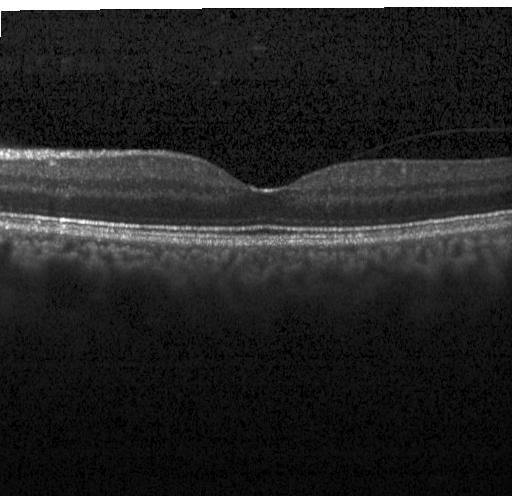

SD-OCT, OCT line scan, through the macula, Heidelberg Spectralis.
Finding: no evidence of CNV, DME, or drusen.